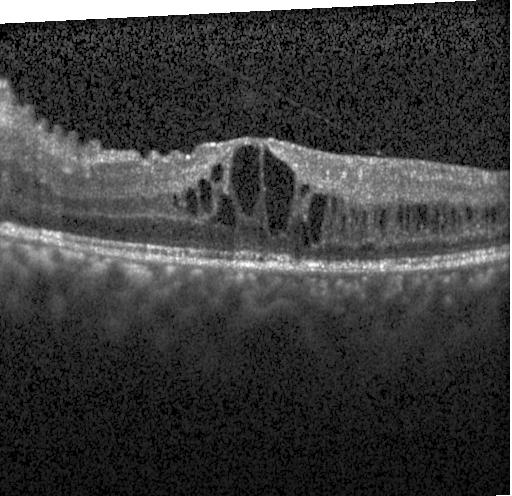
OCT scan showing DME.